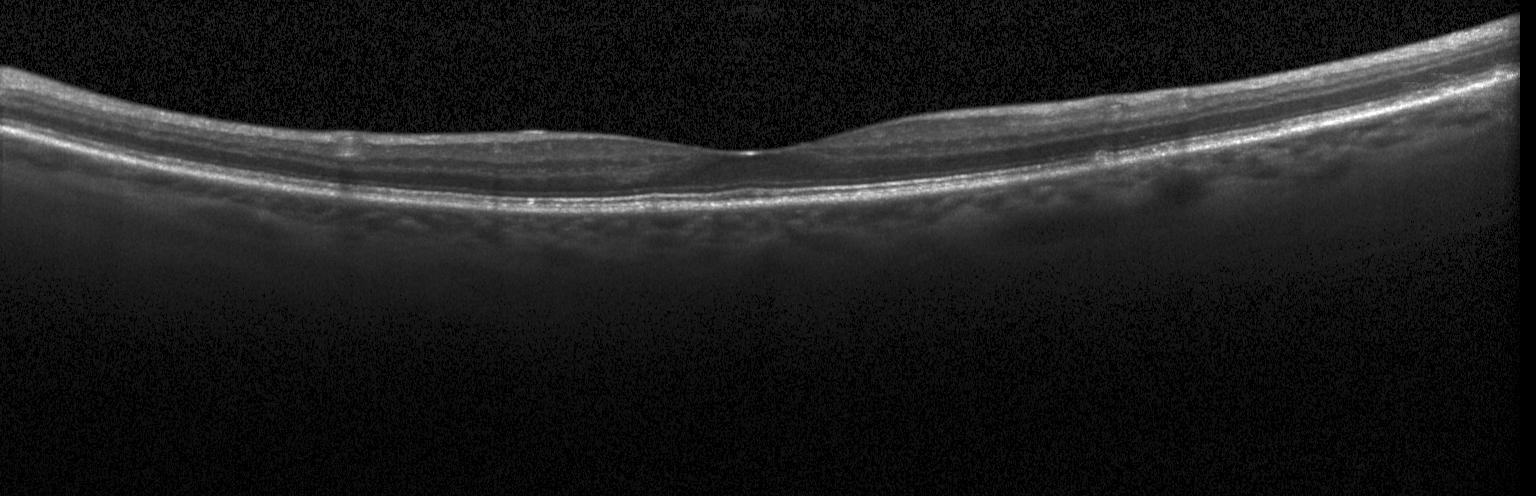 Heidelberg Spectralis; optical coherence tomography B-scan; horizontal scan through the fovea — Assessment: no evidence of choroidal neovascularization, diabetic macular edema, or drusen.